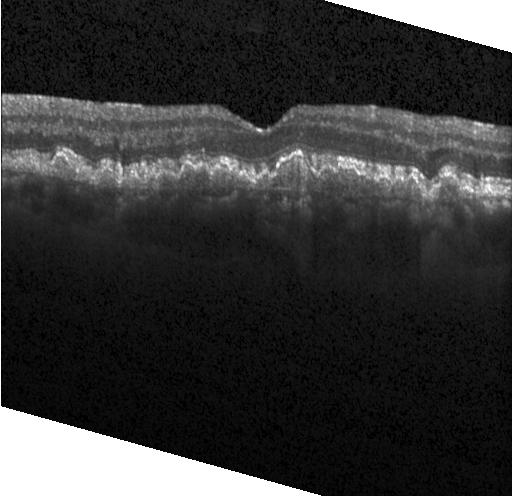 Spectral-domain optical coherence tomography; retinal OCT B-scan; fovea-centered; acquired on a Heidelberg Spectralis. The scan shows choroidal neovascularization (CNV).